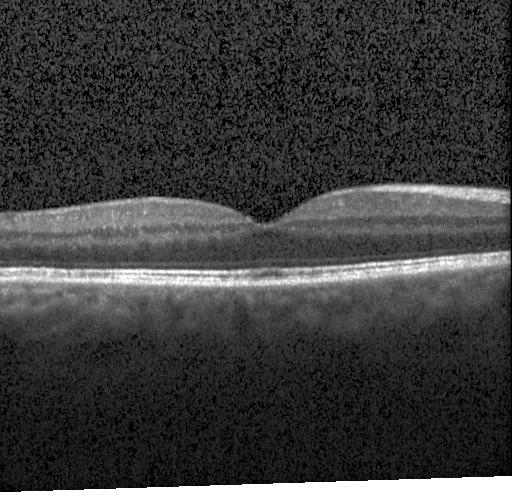 Retinal OCT cross-section — Diagnosis: no choroidal neovascularization, no diabetic macular edema, and no drusen.